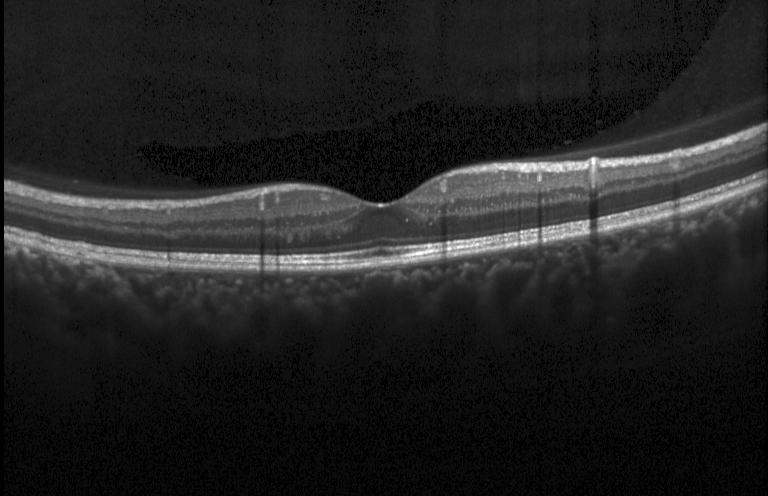
Through the macula. Instrument: Heidelberg Spectralis. Retinal OCT B-scan. Spectral-domain OCT.
Dx: no CNV, DME, or drusen.